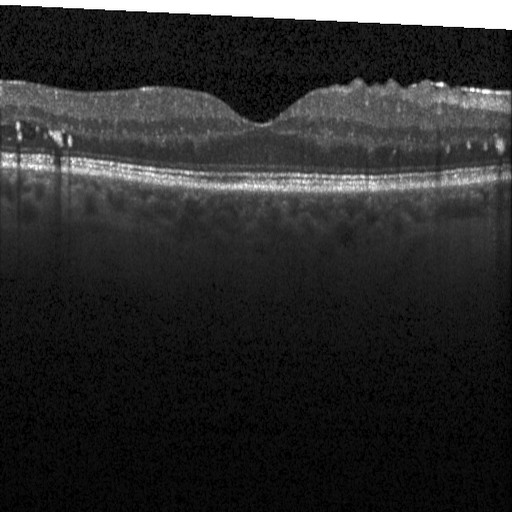
Retinal OCT B-scan — Finding: diabetic macular edema (DME).